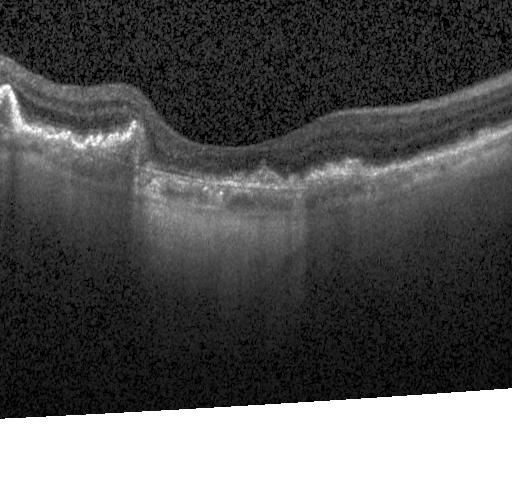

Optical coherence tomography B-scan.
Diagnosis: choroidal neovascularization.